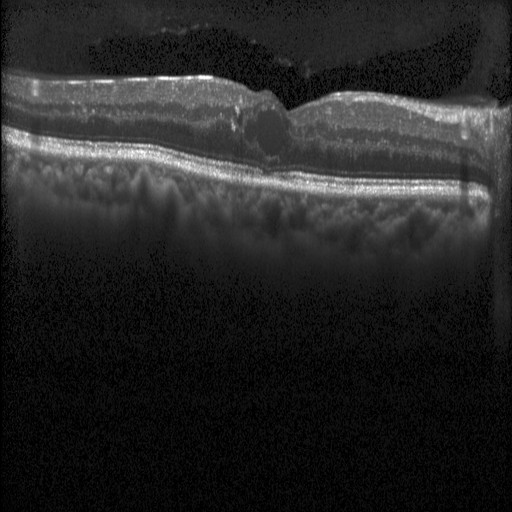 Retinal OCT cross-section showing diabetic macular edema (DME).